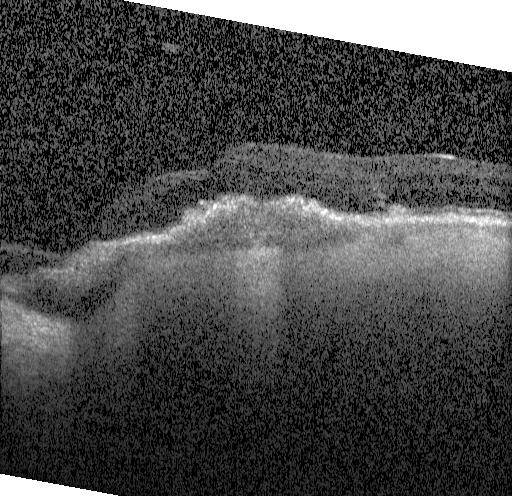 Finding: CNV.